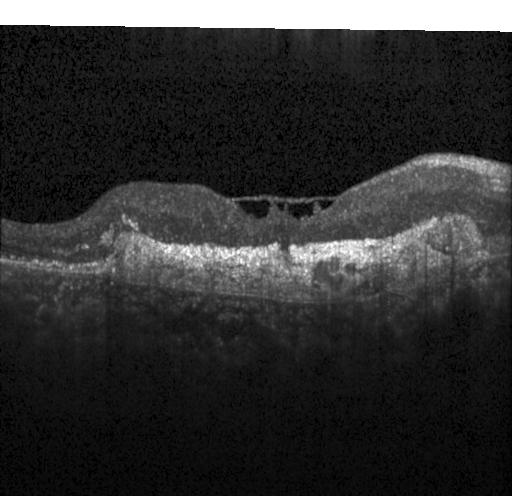
Through the macula, instrument: Heidelberg Spectralis, OCT B-scan.
Impression: a choroidal neovascular membrane.